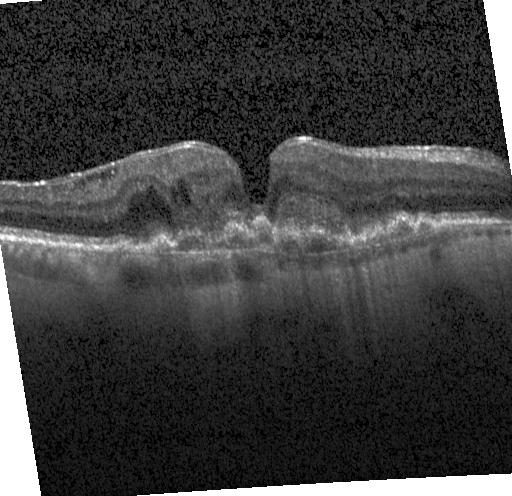 Macular scan, spectral-domain OCT, retinal OCT B-scan
Choroidal neovascularization (CNV).